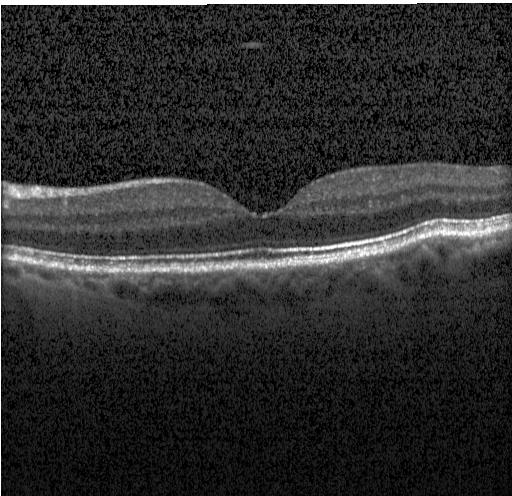 Retinal OCT B-scan; spectral-domain optical coherence tomography. Impression: no evidence of choroidal neovascularization, diabetic macular edema, or drusen.